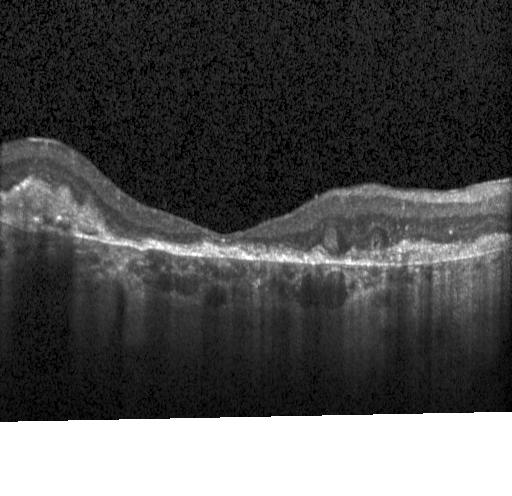
A choroidal neovascular membrane.